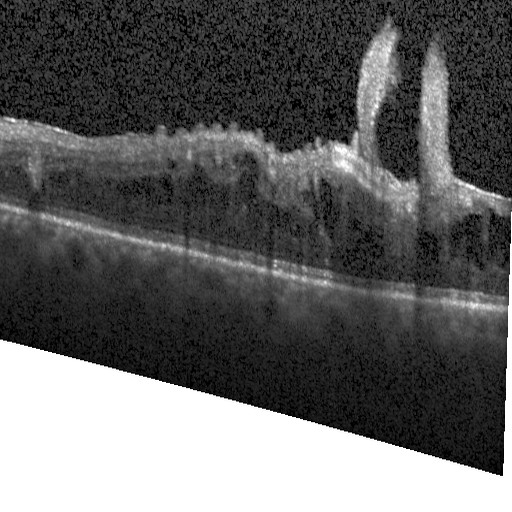
This B-scan demonstrates DME.